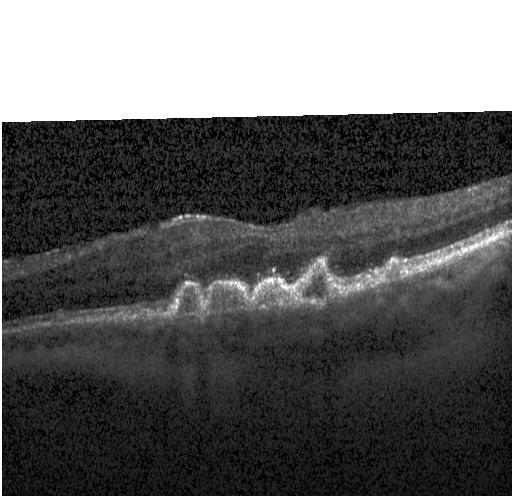
This B-scan demonstrates multiple drusen.